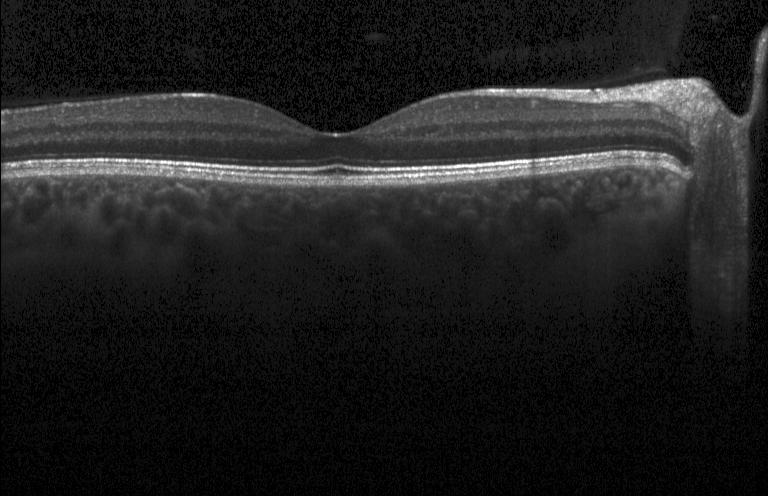

Assessment: neither choroidal neovascularization, diabetic macular edema, nor drusen.